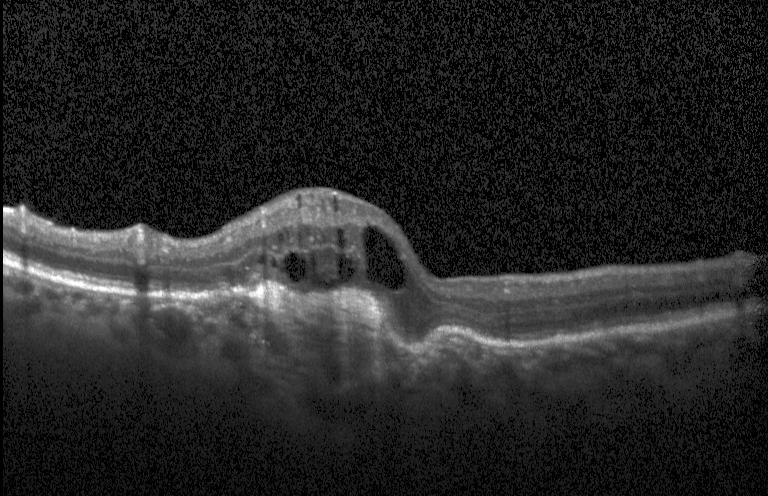 OCT B-scan. Heidelberg Spectralis — Impression: CNV.